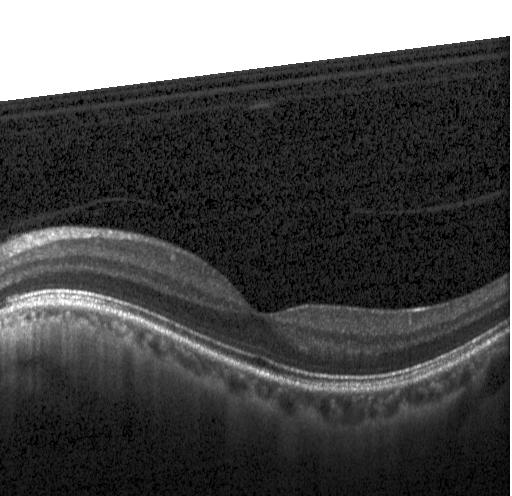

Finding: no choroidal neovascularization, diabetic macular edema, or drusen.